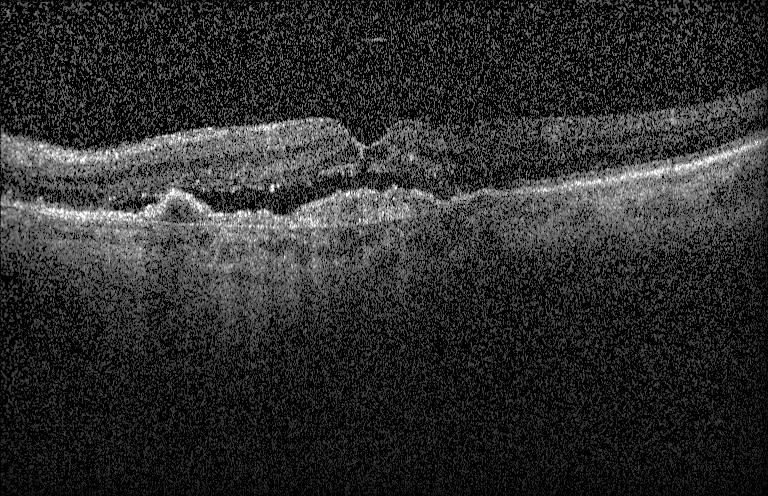 Spectral-domain OCT · horizontal scan through the fovea · retinal OCT B-scan · Heidelberg Spectralis
Dx: CNV.